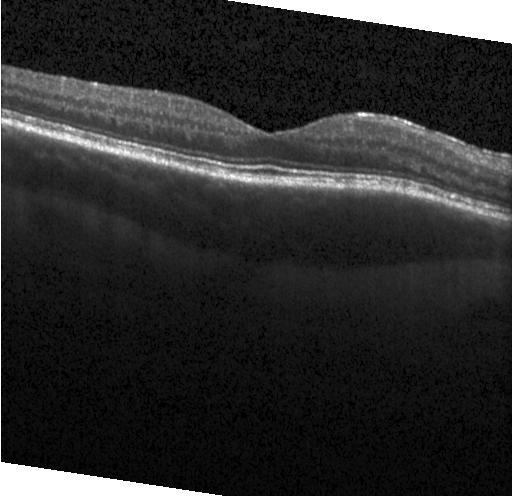 Spectral-domain optical coherence tomography · horizontal scan through the fovea · OCT B-scan · Heidelberg Spectralis. Diagnosis: neither choroidal neovascularization, diabetic macular edema, nor drusen.